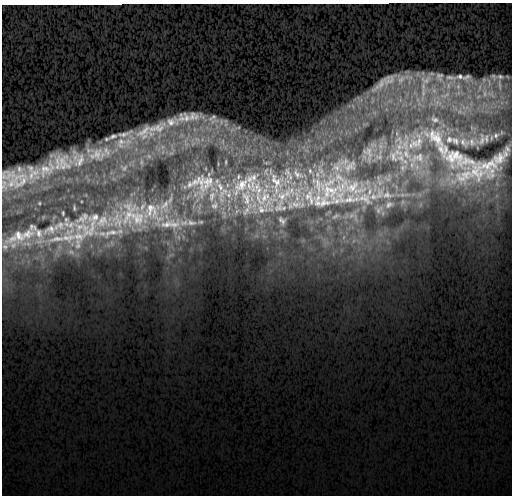 Acquired on a Heidelberg Spectralis, spectral-domain OCT, retinal OCT cross-section
Impression: a choroidal neovascular membrane.